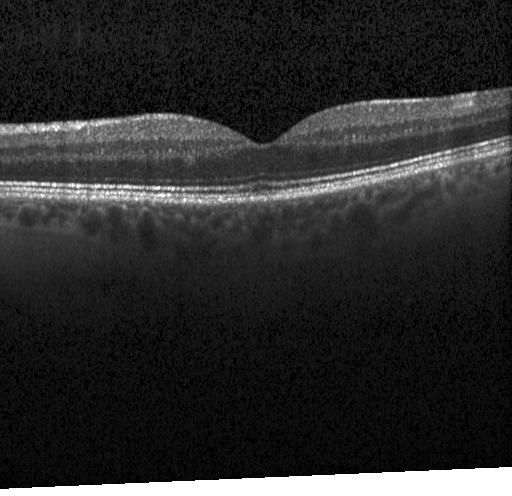 Finding: neither choroidal neovascularization, diabetic macular edema, nor drusen.